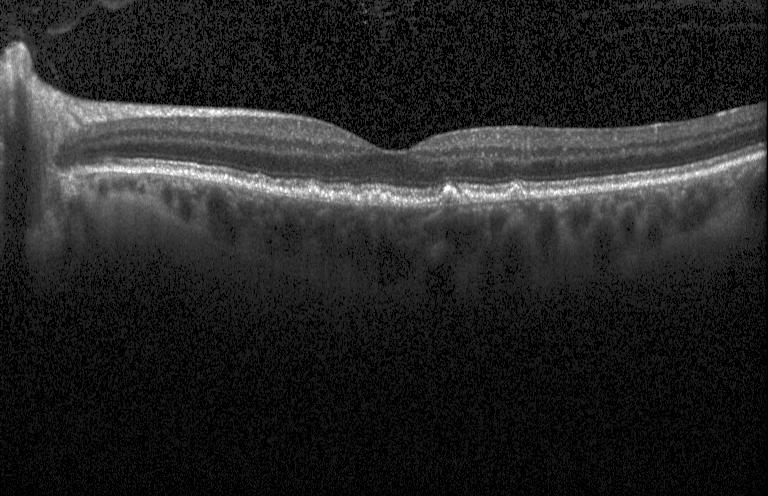
OCT line scan
The scan shows multiple drusen.